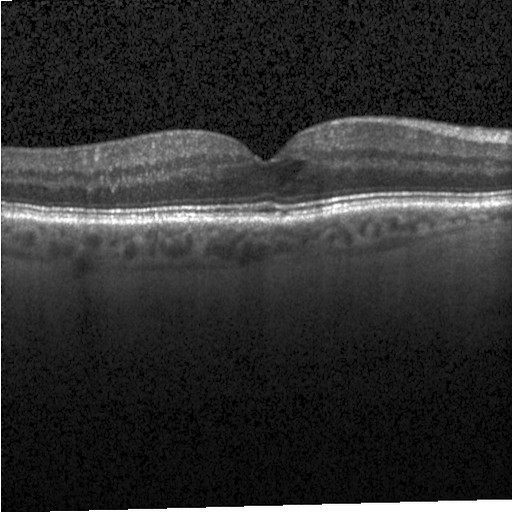 OCT B-scan — Finding: diabetic macular edema.